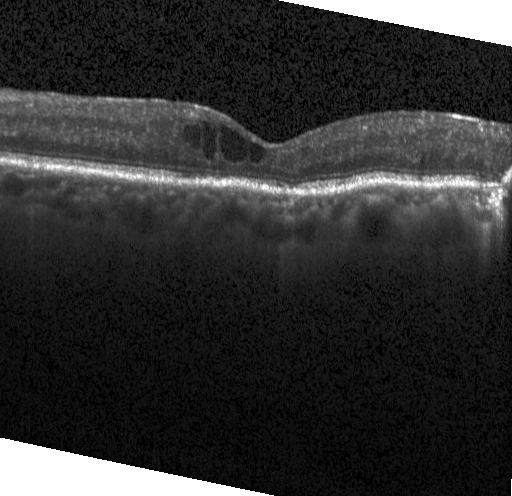
OCT scan showing diabetic macular edema (DME).